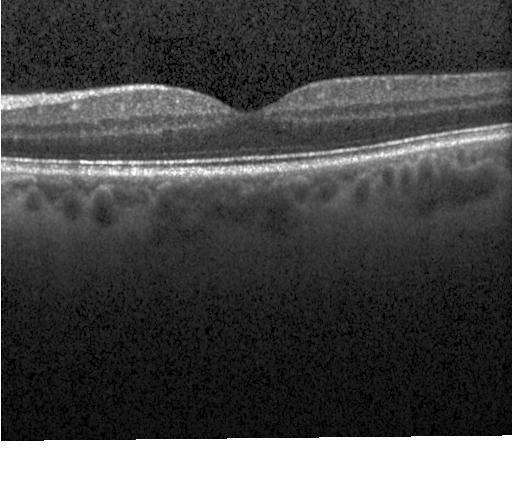

Finding: no choroidal neovascularization, no diabetic macular edema, and no drusen.